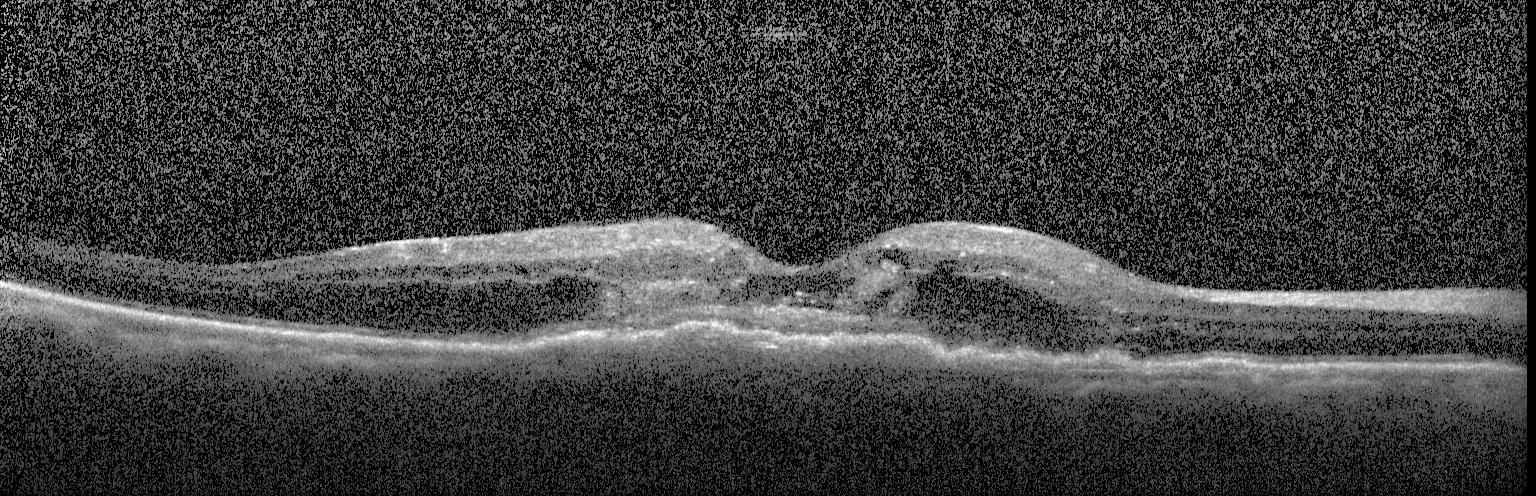
Macular OCT demonstrating choroidal neovascularization (CNV).